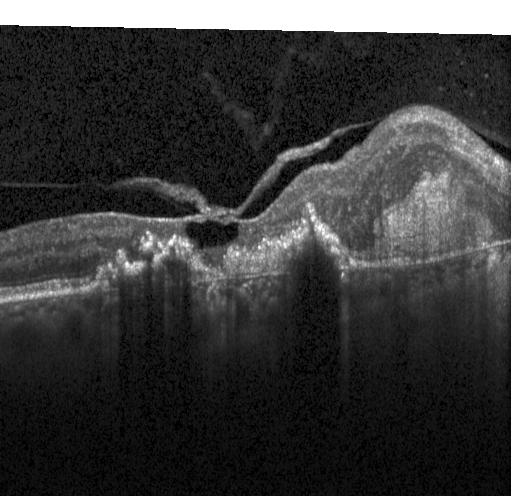

Finding: choroidal neovascularization (CNV).